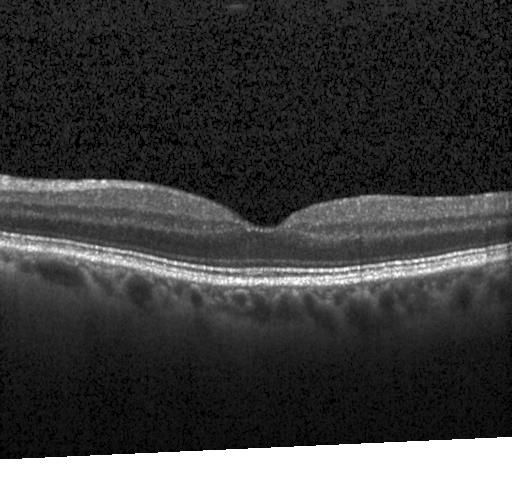
Fovea-centered, acquired on a Heidelberg Spectralis, SD-OCT, OCT line scan. Impression: no choroidal neovascularization, diabetic macular edema, or drusen.